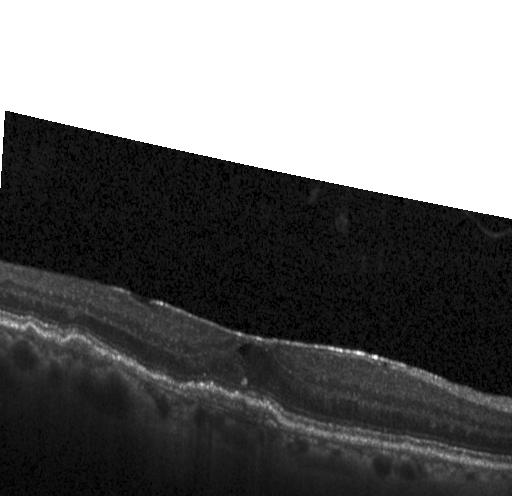

Macular scan · Heidelberg Spectralis · optical coherence tomography B-scan.
Impression: a choroidal neovascular membrane.